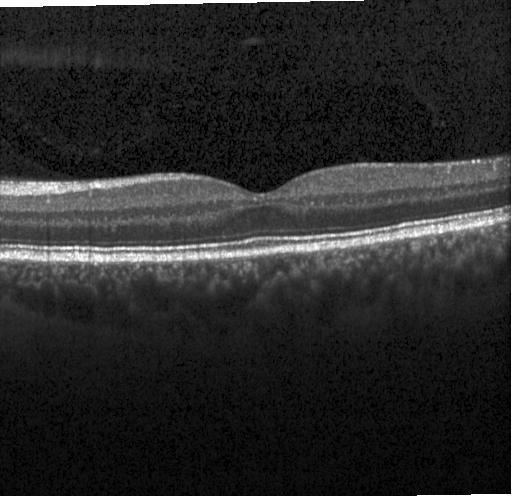 Assessment: no choroidal neovascularization, no diabetic macular edema, and no drusen.